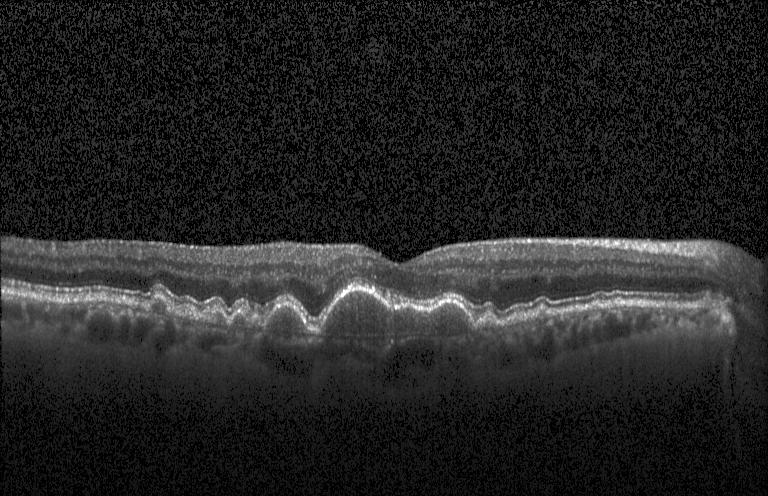

Spectral-domain OCT. Heidelberg Spectralis. Macular scan. OCT B-scan
Impression: sub-RPE drusenoid deposits.